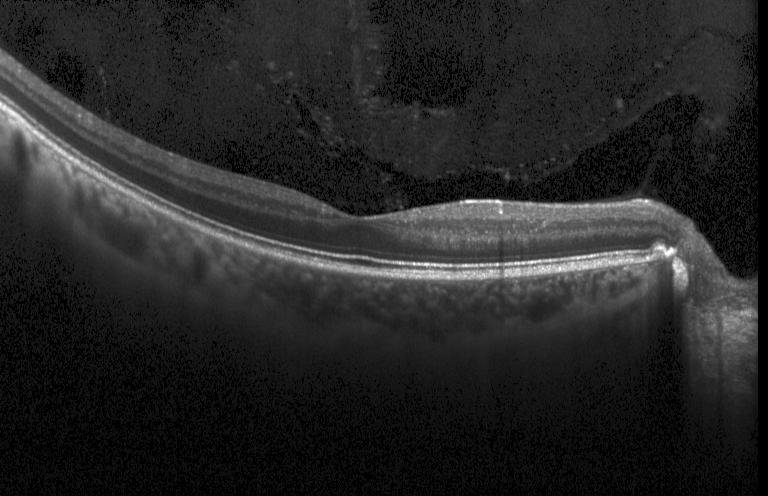
Acquired on a Heidelberg Spectralis, retinal OCT cross-section, SD-OCT, fovea-centered.
Dx: neither choroidal neovascularization, diabetic macular edema, nor drusen.